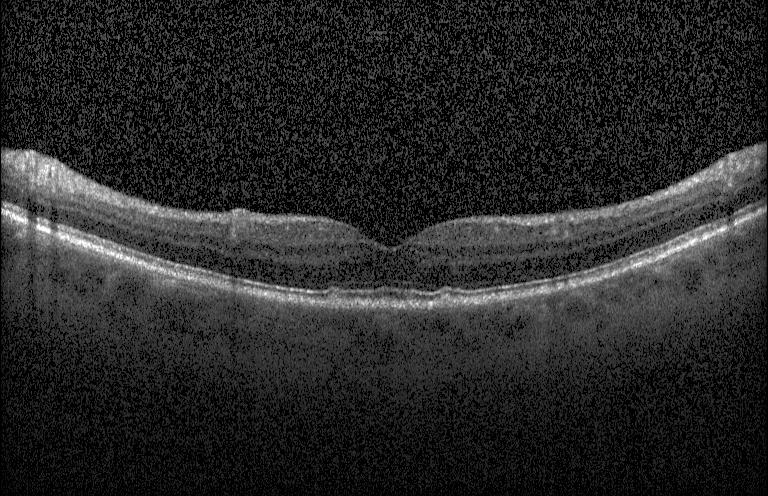 Finding: multiple drusen.